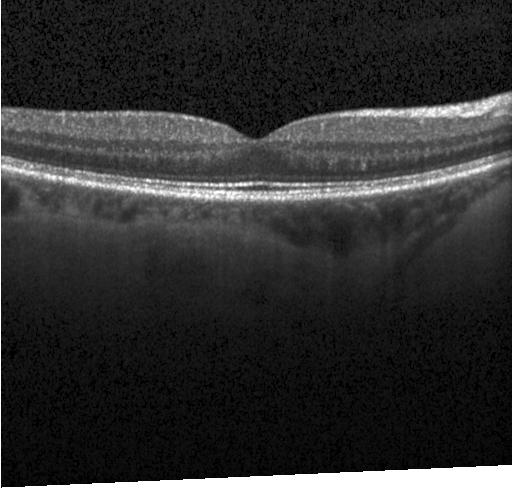
Horizontal scan through the fovea. Heidelberg Spectralis. Retinal OCT B-scan.
Finding: no choroidal neovascularization, no diabetic macular edema, and no drusen.